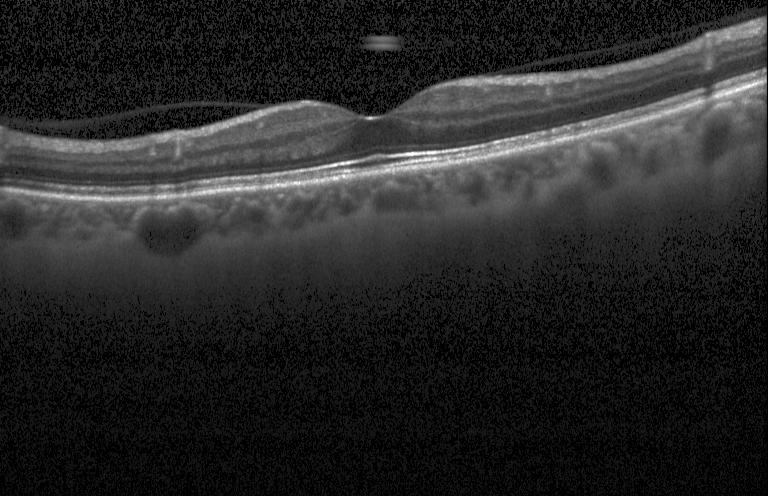
Instrument: Heidelberg Spectralis; OCT B-scan; spectral-domain optical coherence tomography. Macular OCT: no evidence of choroidal neovascularization, diabetic macular edema, or drusen.